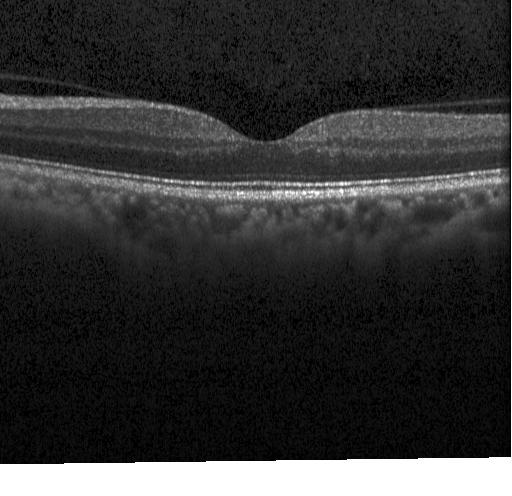 Macular scan, retinal OCT B-scan — OCT finding: neither CNV, DME, nor drusen.